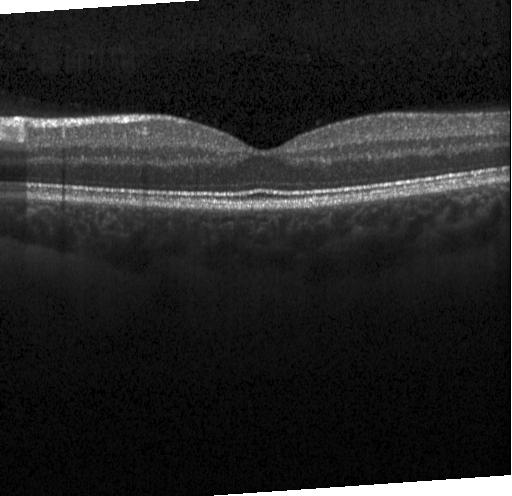

Diagnosis: no evidence of choroidal neovascularization, diabetic macular edema, or drusen.